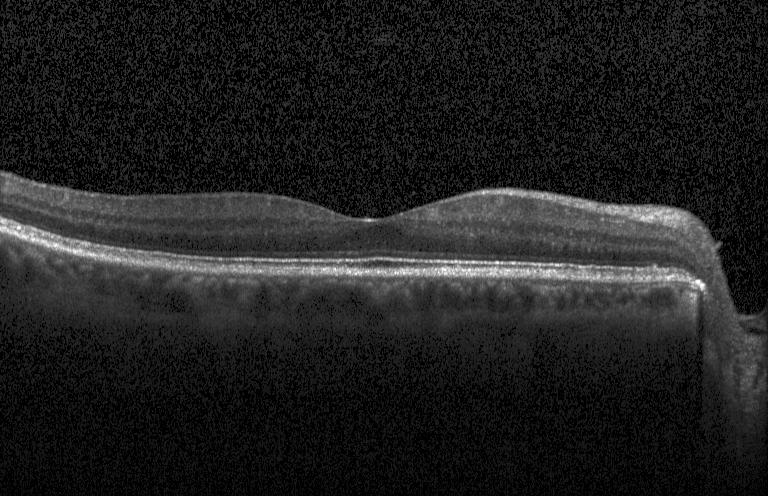

OCT B-scan. Diagnosis: no CNV, DME, or drusen.